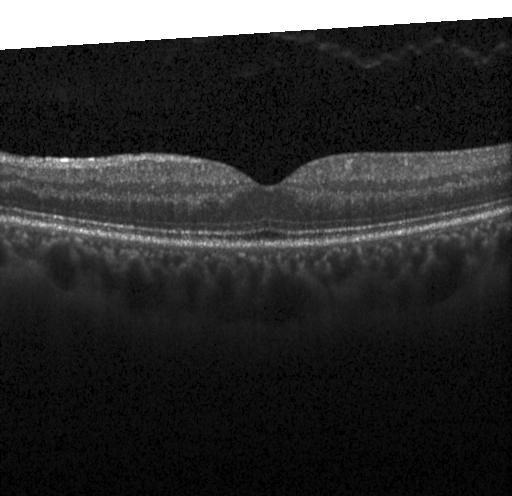 Diagnosis: no evidence of CNV, DME, or drusen.